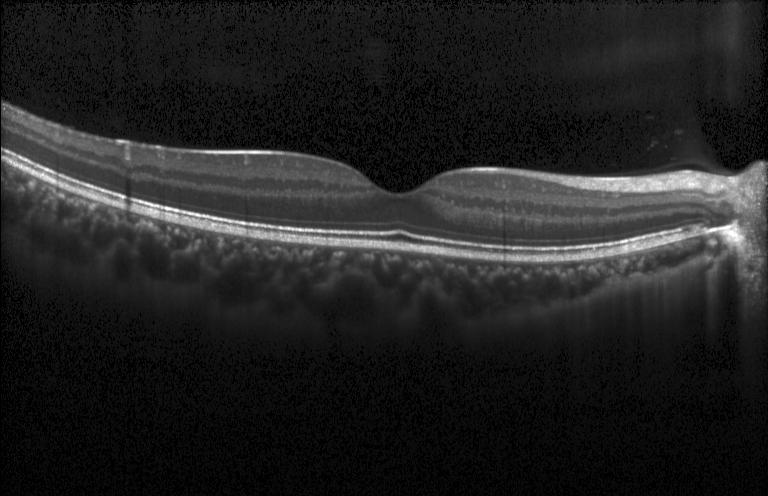

Spectral-domain optical coherence tomography. Optical coherence tomography B-scan. Heidelberg Spectralis OCT system — Diagnosis: no evidence of choroidal neovascularization, diabetic macular edema, or drusen.